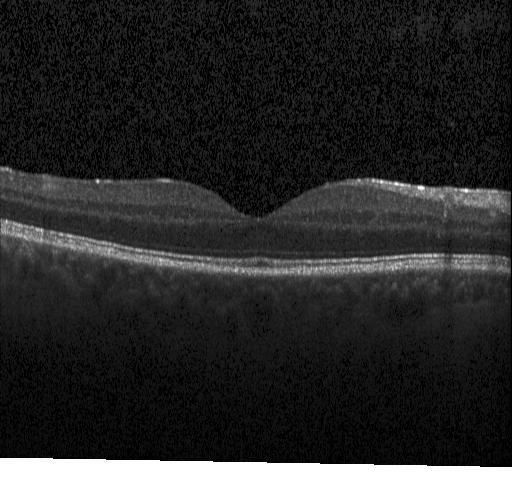

Retinal OCT cross-section · horizontal scan through the fovea. The scan shows no choroidal neovascularization, diabetic macular edema, or drusen.